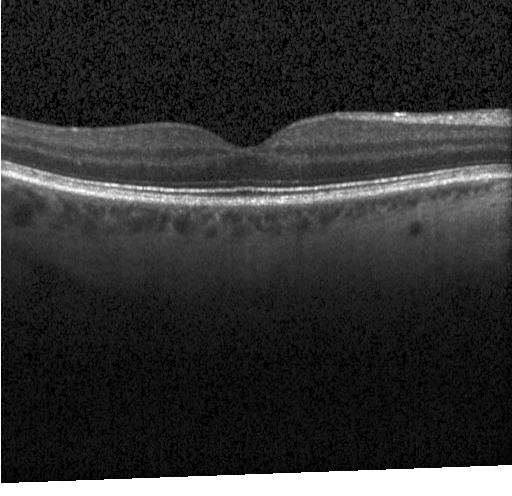

Through the macula · spectral-domain OCT · OCT line scan · acquired on a Heidelberg Spectralis — OCT finding: no CNV, DME, or drusen.